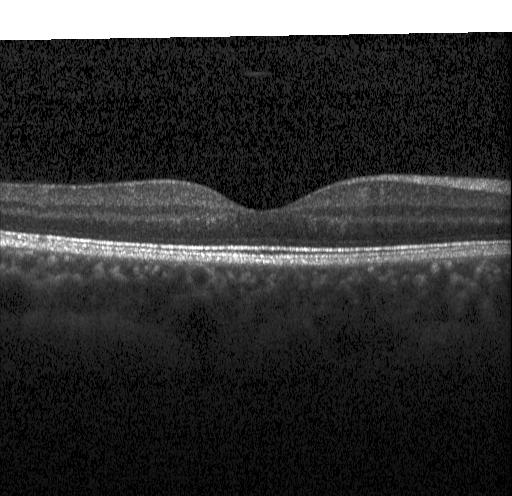

Retinal OCT B-scan
OCT finding: neither CNV, DME, nor drusen.